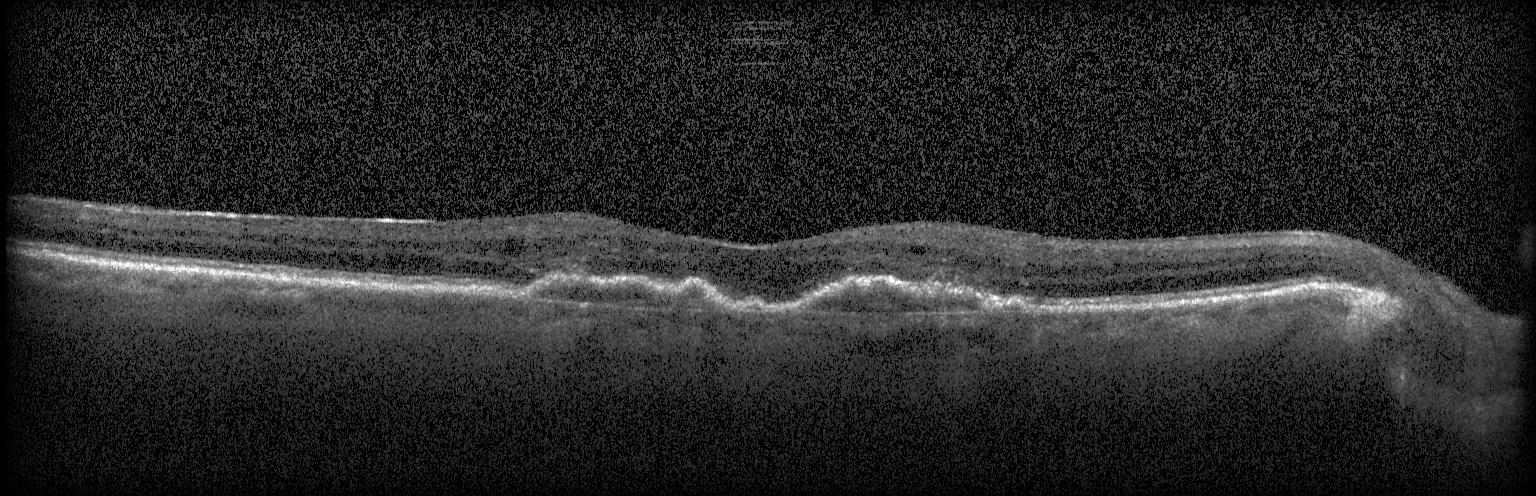

OCT scan showing choroidal neovascularization.